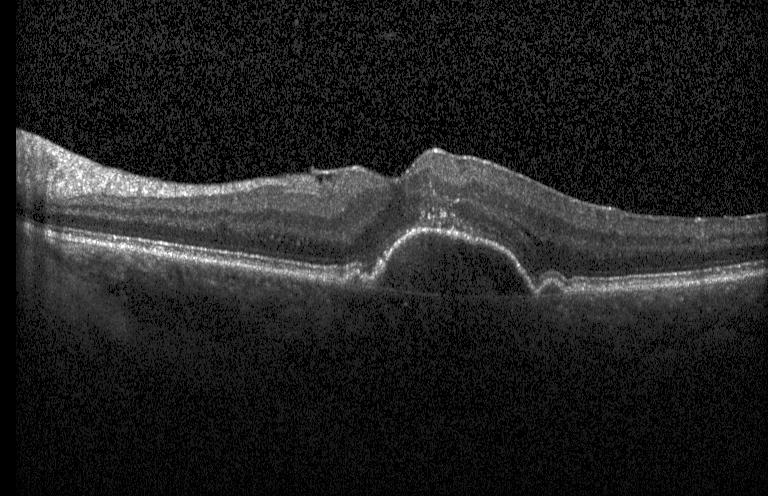

OCT B-scan · macular scan · spectral-domain OCT.
Dx: a choroidal neovascular membrane.